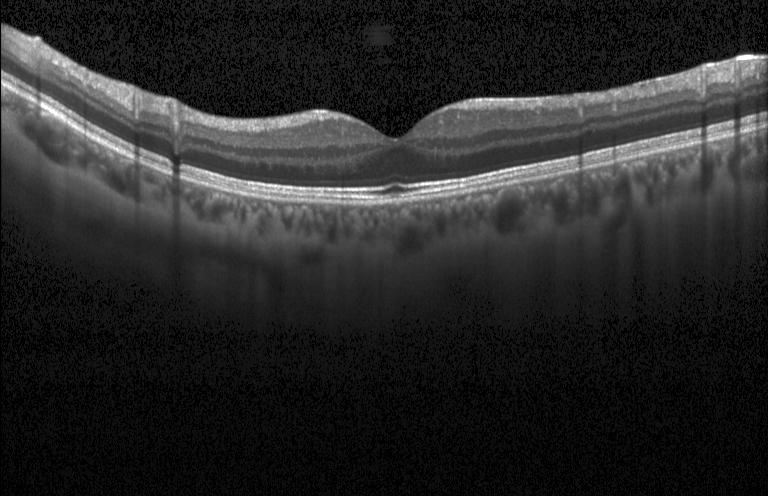

Macular OCT: neither CNV, DME, nor drusen.